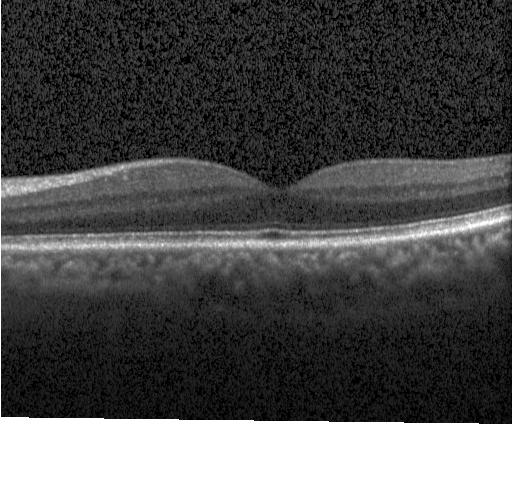
OCT B-scan showing neither choroidal neovascularization, diabetic macular edema, nor drusen.